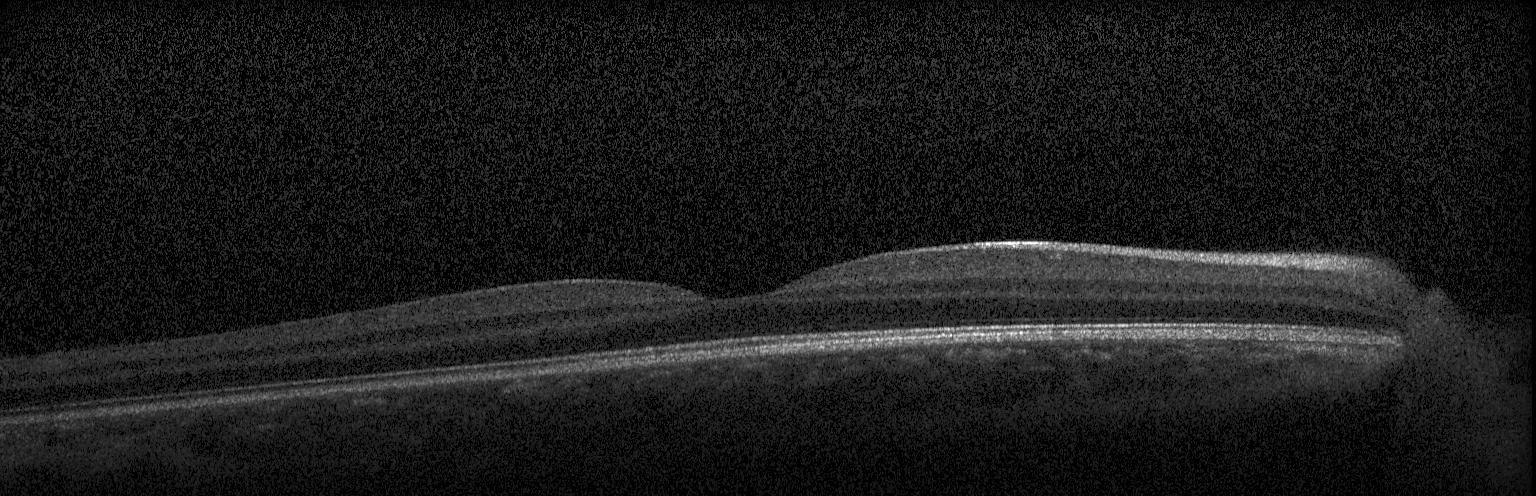

Spectral-domain optical coherence tomography. Retinal OCT cross-section. Assessment: no choroidal neovascularization, diabetic macular edema, or drusen.